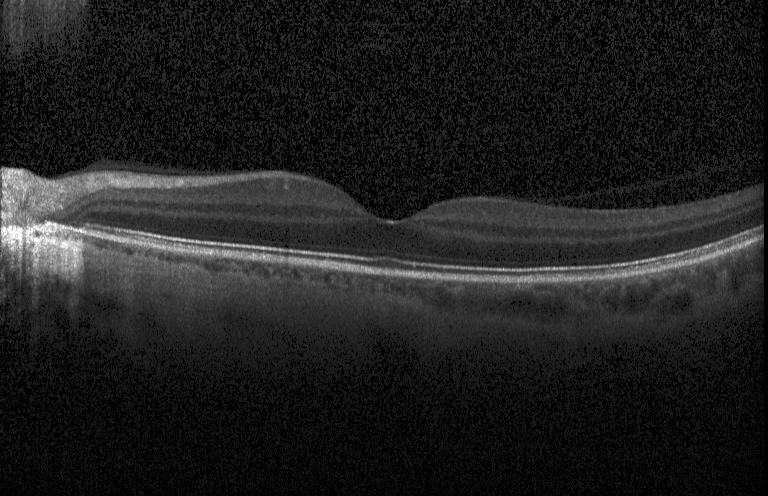 Heidelberg Spectralis; macular scan; OCT line scan
The scan shows no choroidal neovascularization, diabetic macular edema, or drusen.